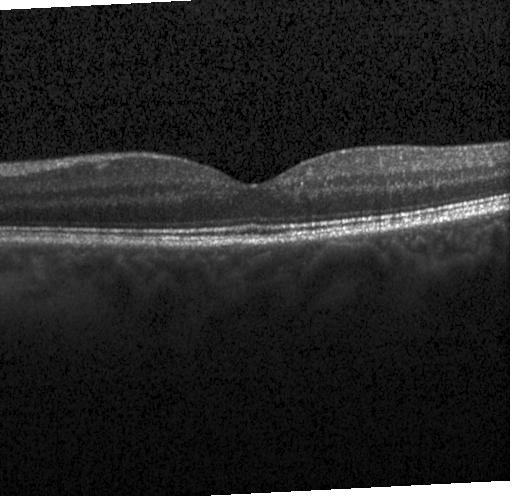 Finding: no CNV, no DME, and no drusen.